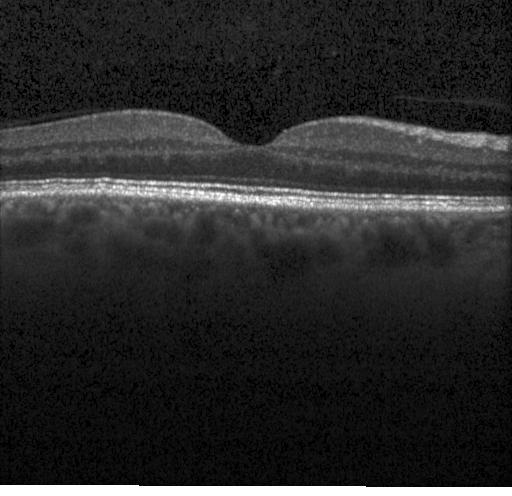

OCT finding: neither CNV, DME, nor drusen.